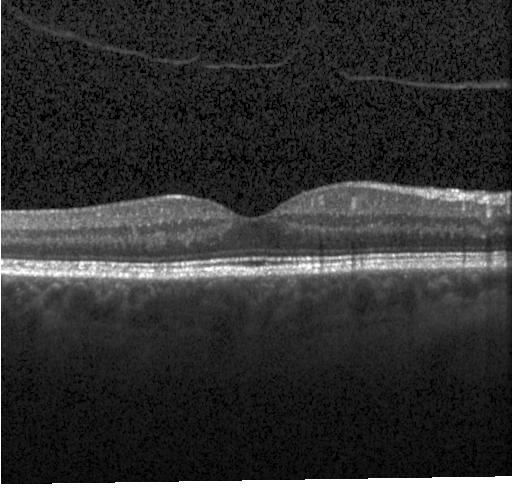
Assessment: no CNV, DME, or drusen.